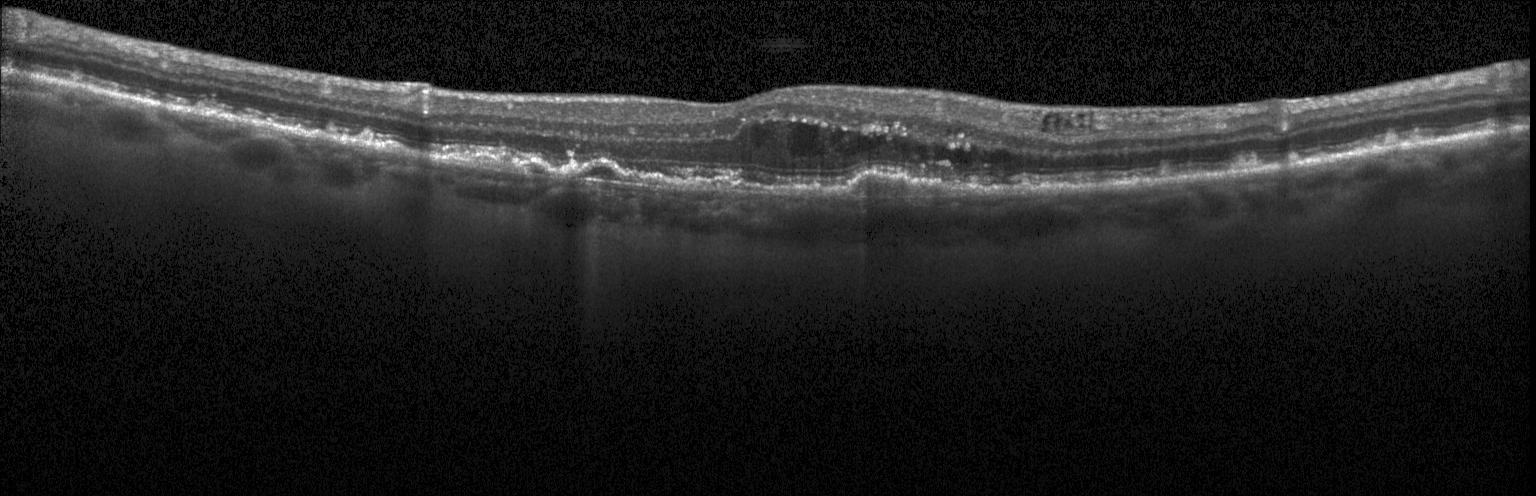

Optical coherence tomography B-scan; instrument: Heidelberg Spectralis; SD-OCT — Macular OCT: a choroidal neovascular membrane.